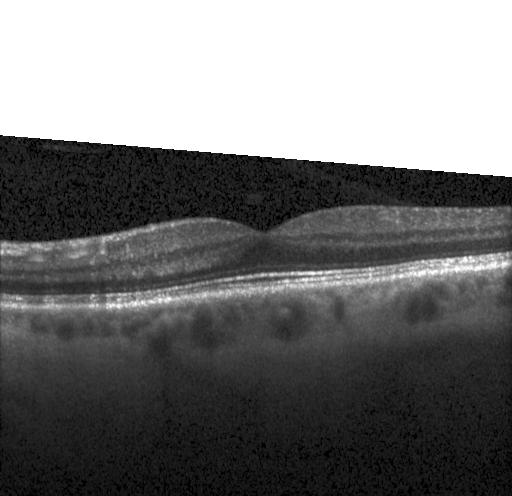 Diagnosis: no CNV, no DME, and no drusen.